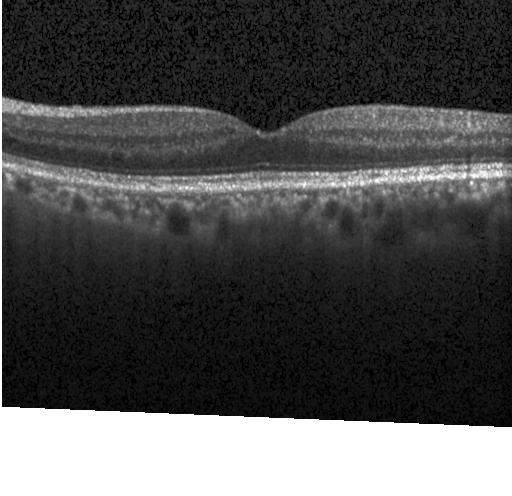
Retinal OCT B-scan, acquired on a Heidelberg Spectralis.
Finding: no evidence of choroidal neovascularization, diabetic macular edema, or drusen.